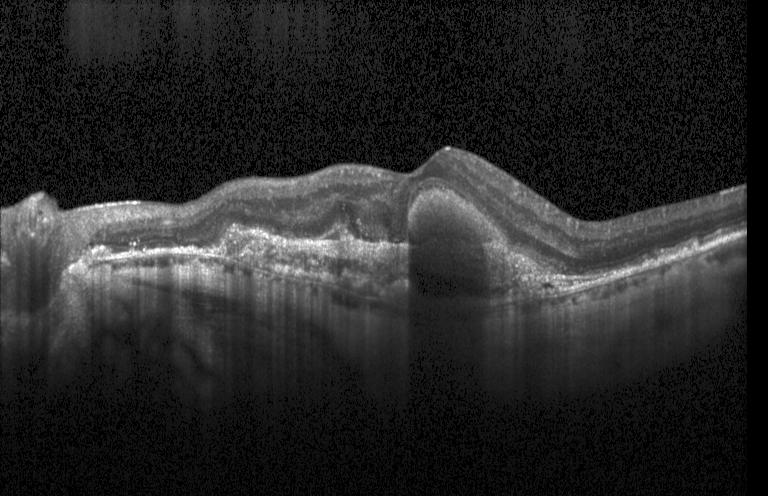
Choroidal neovascularization (CNV).